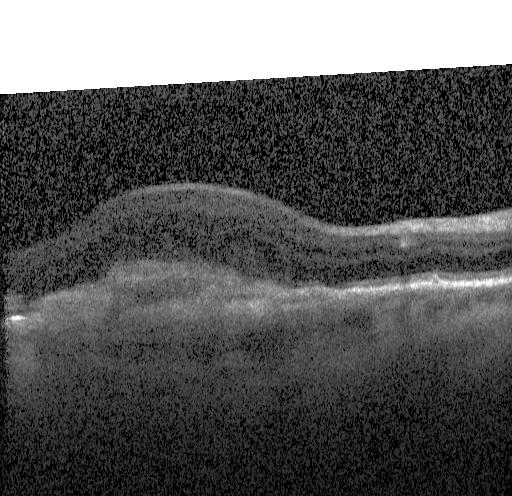
Optical coherence tomography B-scan · SD-OCT
OCT finding: a choroidal neovascular membrane.